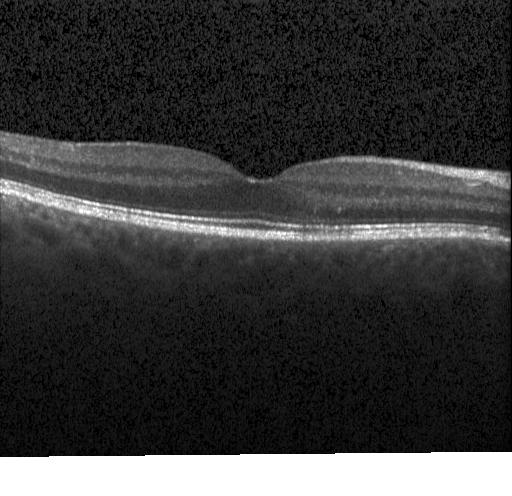 Finding: no evidence of choroidal neovascularization, diabetic macular edema, or drusen.